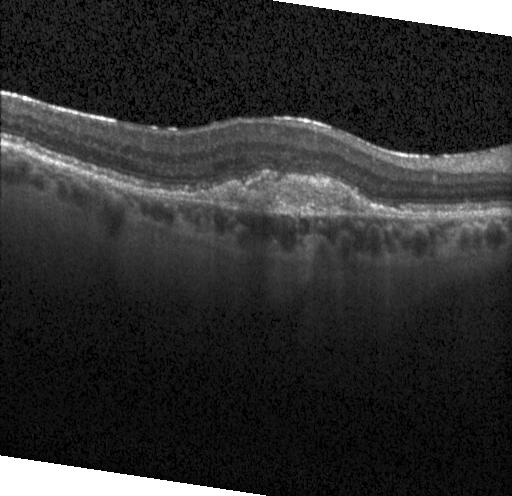 Dx: a choroidal neovascular membrane.